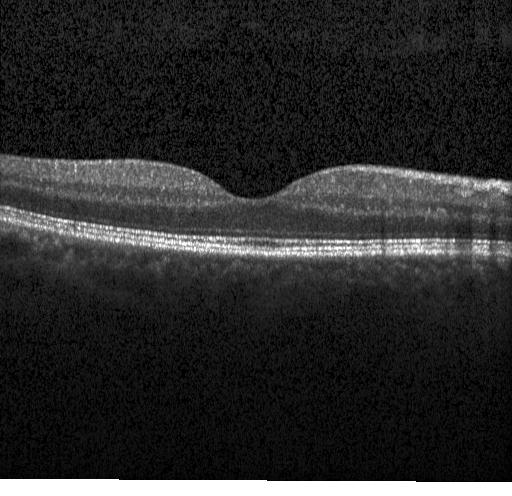

Retinal OCT B-scan · centered on the fovea.
Finding: neither CNV, DME, nor drusen.